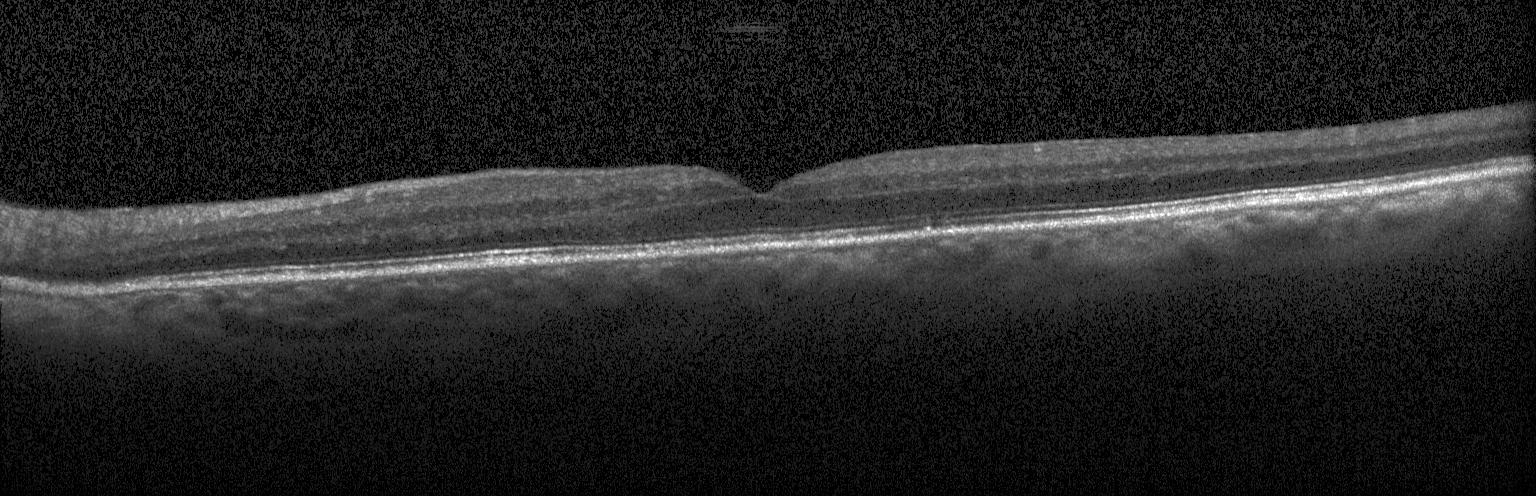

Diagnosis: no choroidal neovascularization, diabetic macular edema, or drusen.